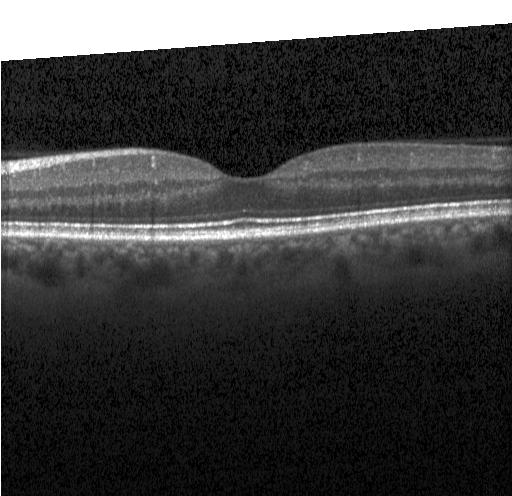 Retinal OCT cross-section.
Finding: neither CNV, DME, nor drusen.